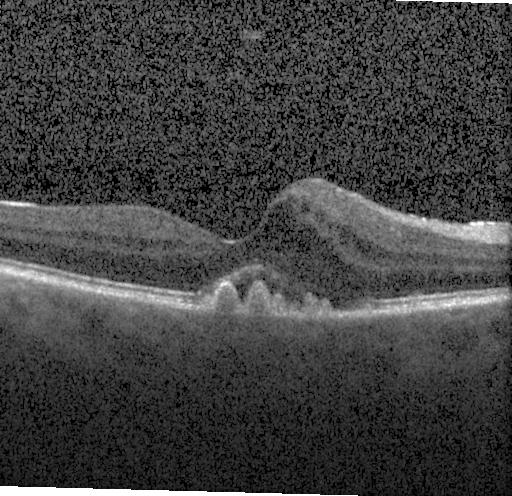
Diagnosis: a choroidal neovascular membrane.